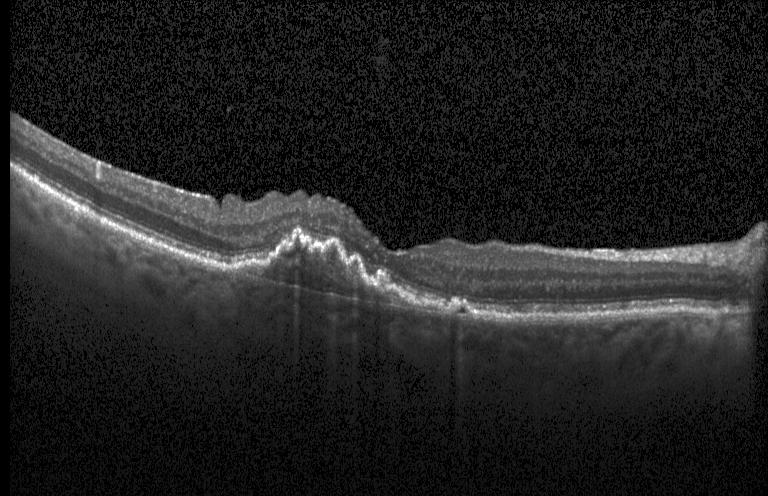 Assessment: a choroidal neovascular membrane.